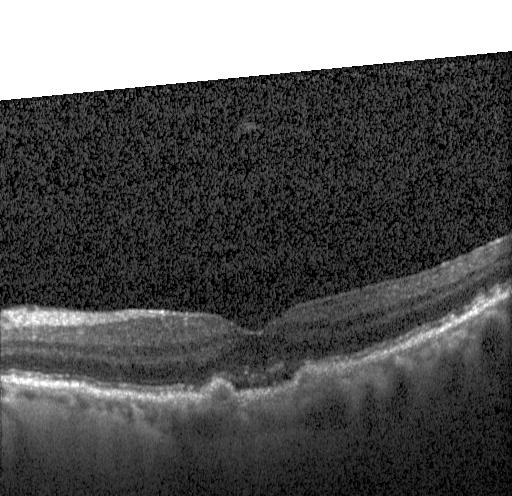
Retinal OCT cross-section; Heidelberg Spectralis; through the macula; spectral-domain optical coherence tomography.
Macular OCT: a choroidal neovascular membrane.